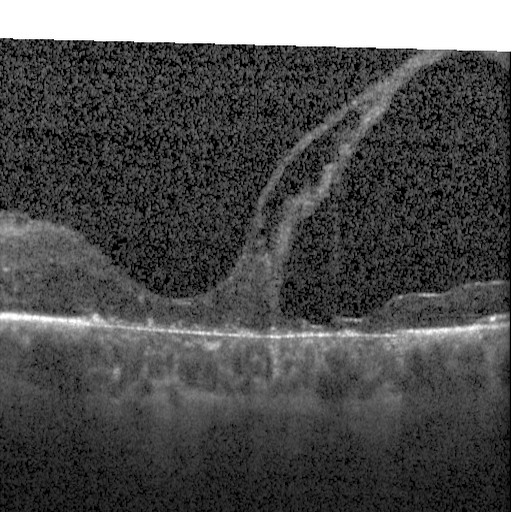
Finding: diabetic macular edema.